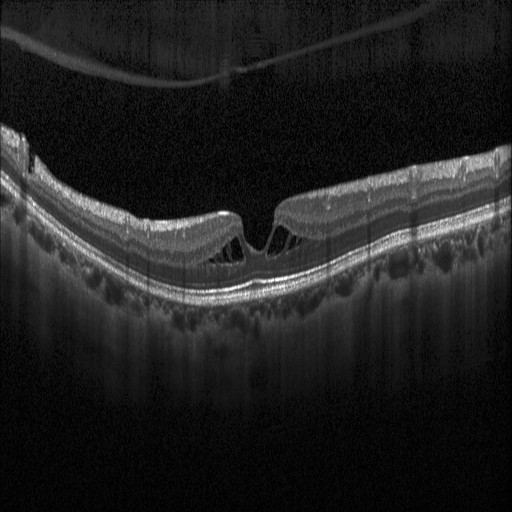 SD-OCT. Retinal OCT cross-section
Diagnosis: DME.